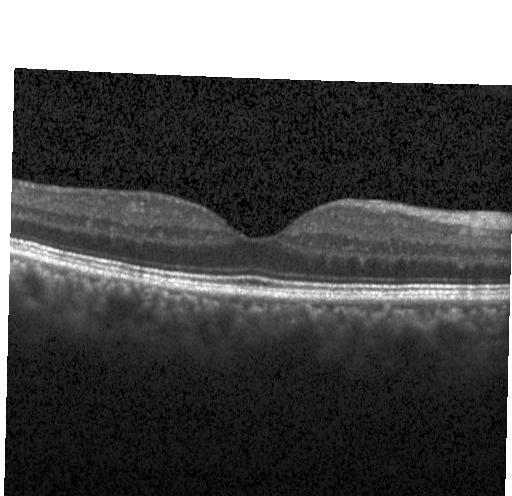
OCT line scan, centered on the fovea, spectral-domain OCT.
Assessment: no evidence of choroidal neovascularization, diabetic macular edema, or drusen.